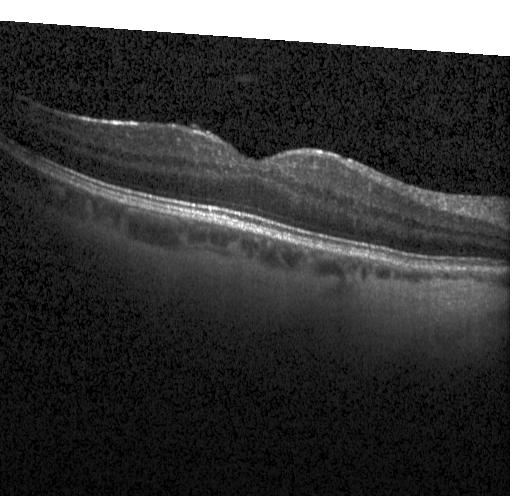

Spectral-domain OCT. Retinal OCT B-scan. Instrument: Heidelberg Spectralis. Fovea-centered — Diagnosis: neither CNV, DME, nor drusen.